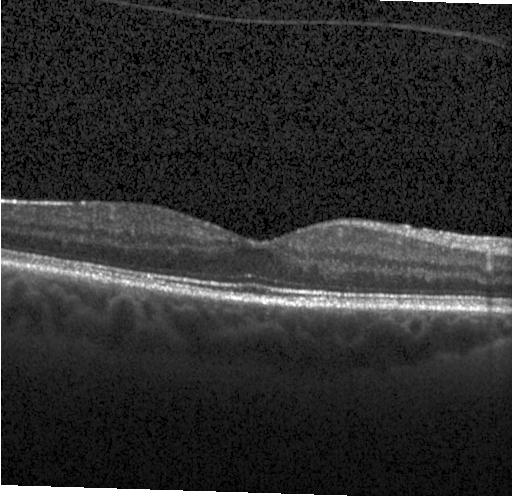 Finding: no CNV, no DME, and no drusen.